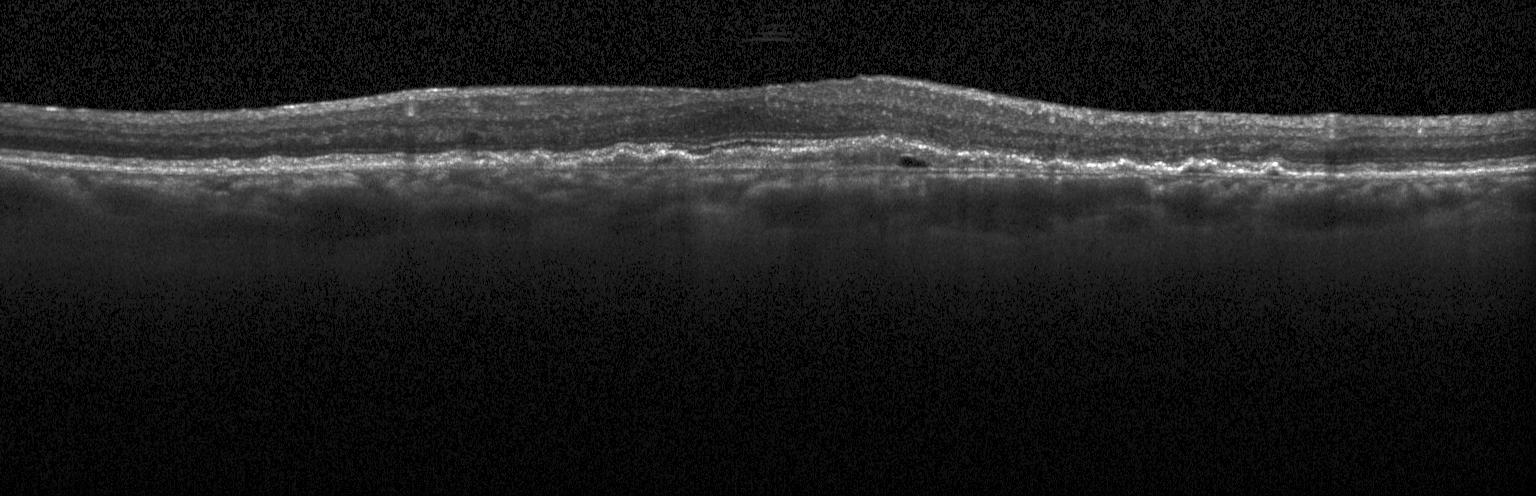
Optical coherence tomography scan. Impression: choroidal neovascularization.